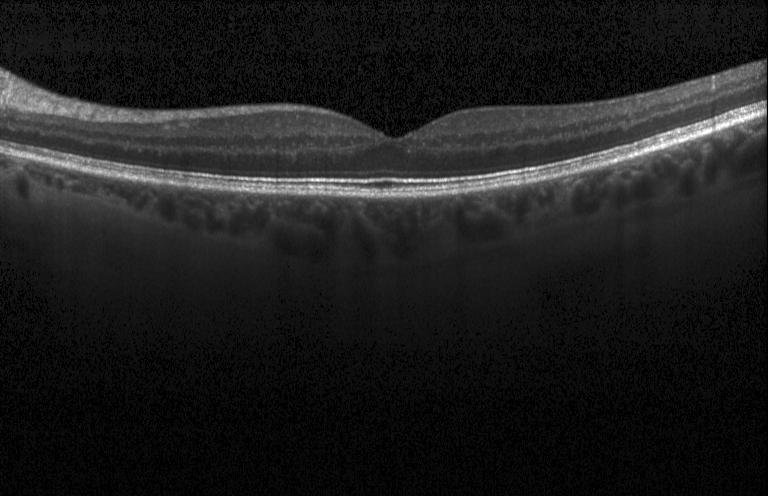

Spectral-domain OCT, retinal OCT B-scan, Heidelberg Spectralis OCT system.
Macular OCT: no evidence of choroidal neovascularization, diabetic macular edema, or drusen.